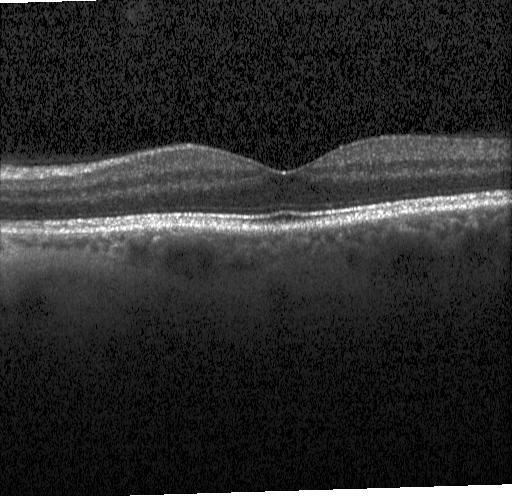

Horizontal scan through the fovea; retinal OCT cross-section; Heidelberg Spectralis — Impression: no choroidal neovascularization, diabetic macular edema, or drusen.